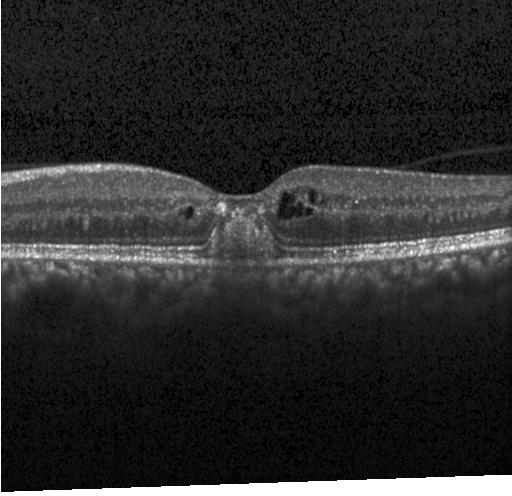 OCT B-scan · Heidelberg Spectralis OCT system.
The scan shows a choroidal neovascular membrane.